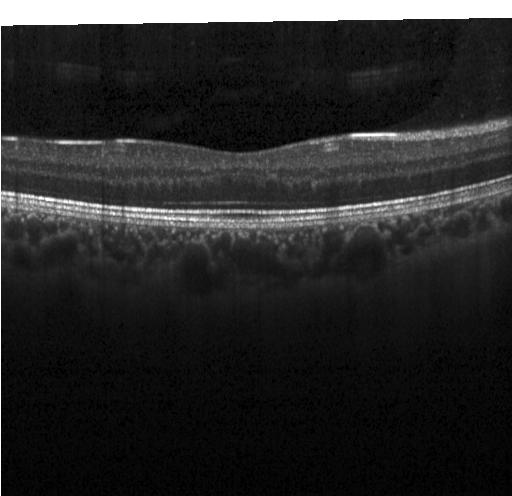
Macular OCT: no choroidal neovascularization, diabetic macular edema, or drusen.